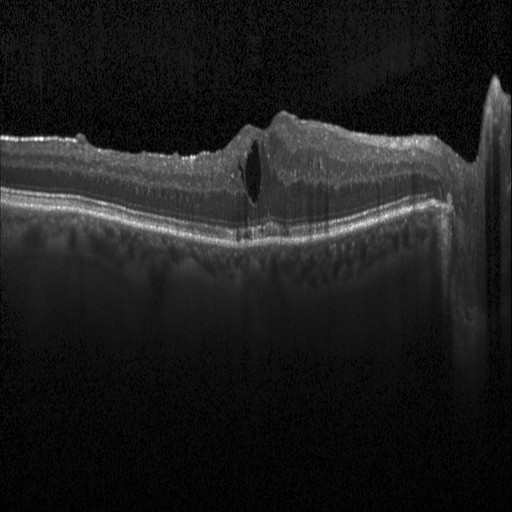 Finding: DME.